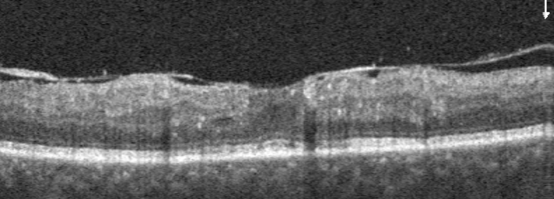 Retinal OCT cross-section. Through the macula. Acquired on an Optovue Avanti RTVue XR
Finding: diabetic macular edema.